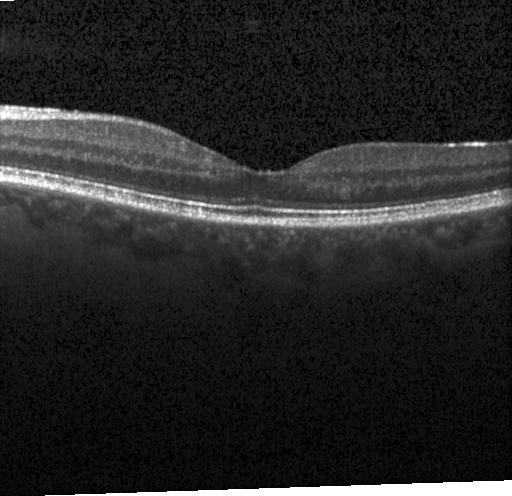 Macular OCT demonstrating no choroidal neovascularization, no diabetic macular edema, and no drusen.